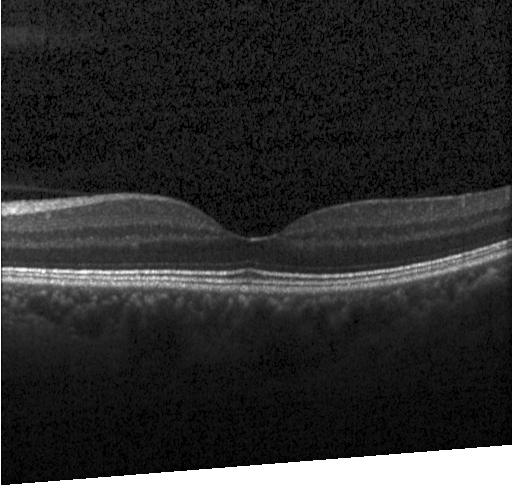

Horizontal scan through the fovea; retinal OCT cross-section; acquired on a Heidelberg Spectralis.
Diagnosis: neither CNV, DME, nor drusen.